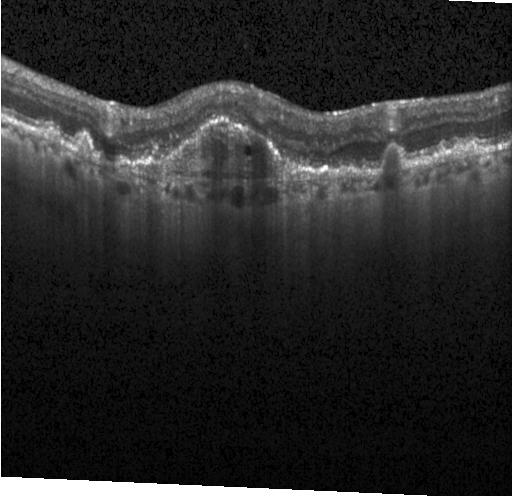

Horizontal scan through the fovea, spectral-domain optical coherence tomography, retinal OCT cross-section, Heidelberg Spectralis.
CNV.